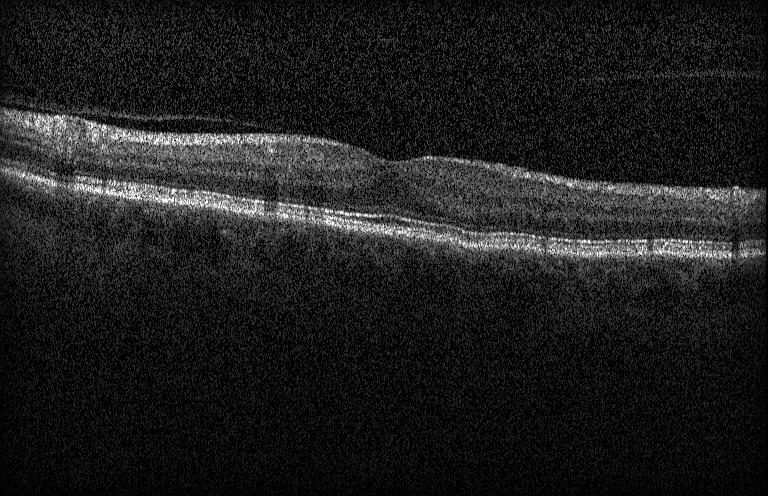

Impression: no choroidal neovascularization, diabetic macular edema, or drusen.